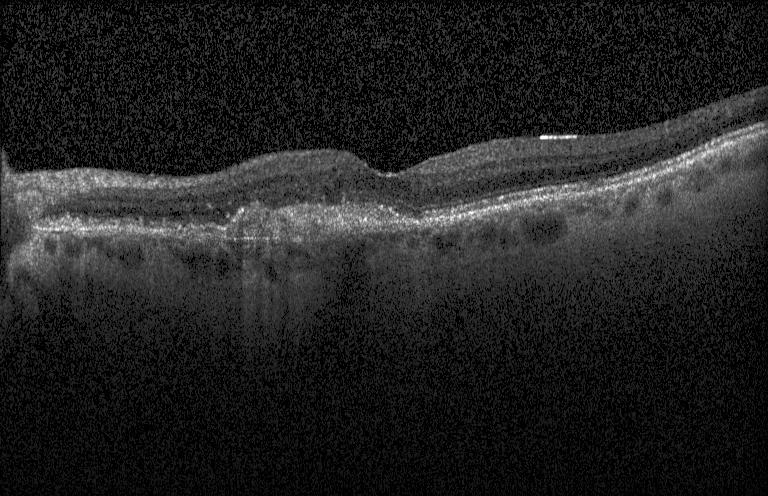

OCT B-scan showing a choroidal neovascular membrane.